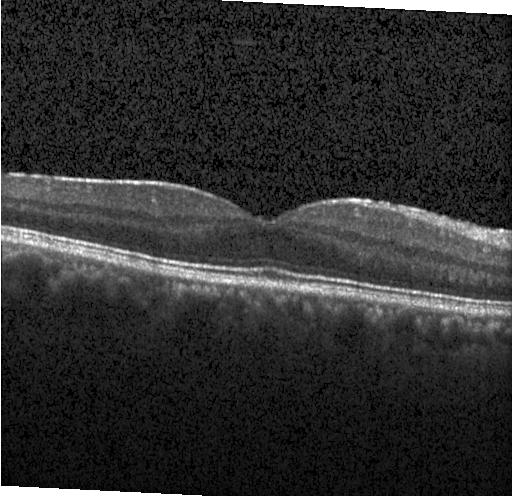
OCT B-scan. Macular OCT: neither choroidal neovascularization, diabetic macular edema, nor drusen.